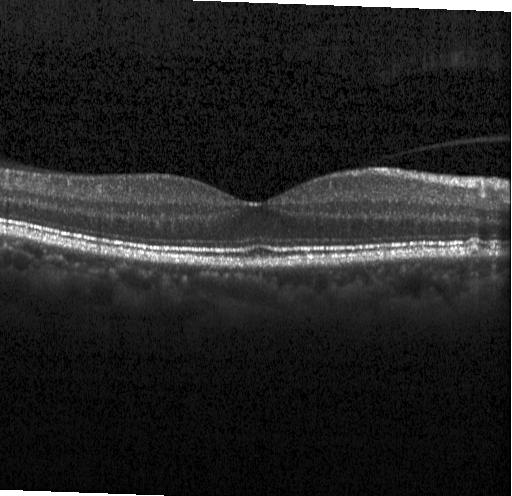 Heidelberg Spectralis, centered on the fovea, optical coherence tomography scan, spectral-domain optical coherence tomography.
Finding: no choroidal neovascularization, diabetic macular edema, or drusen.